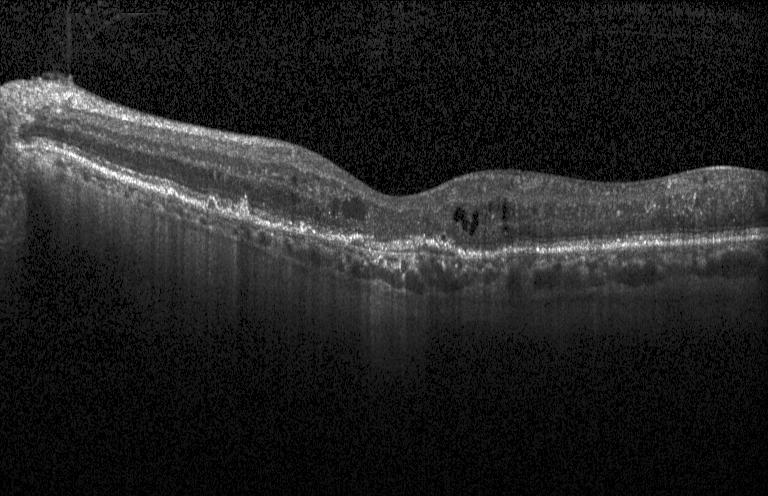 Centered on the fovea; OCT B-scan; spectral-domain optical coherence tomography. Dx: CNV.